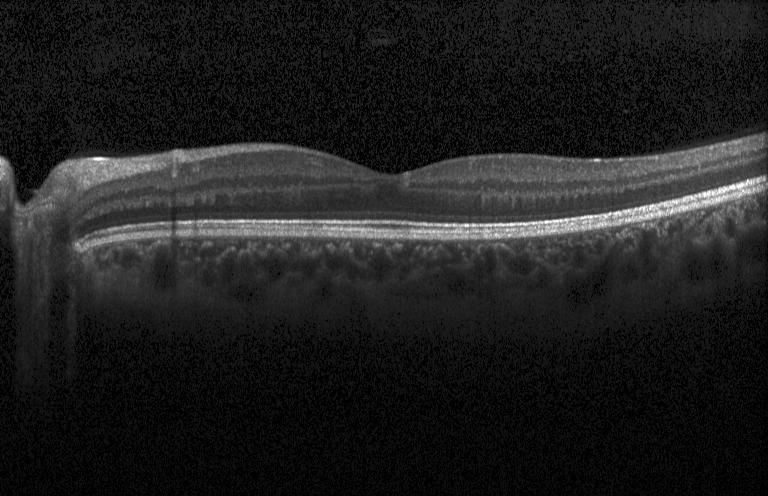 Retinal OCT B-scan.
The scan shows neither choroidal neovascularization, diabetic macular edema, nor drusen.